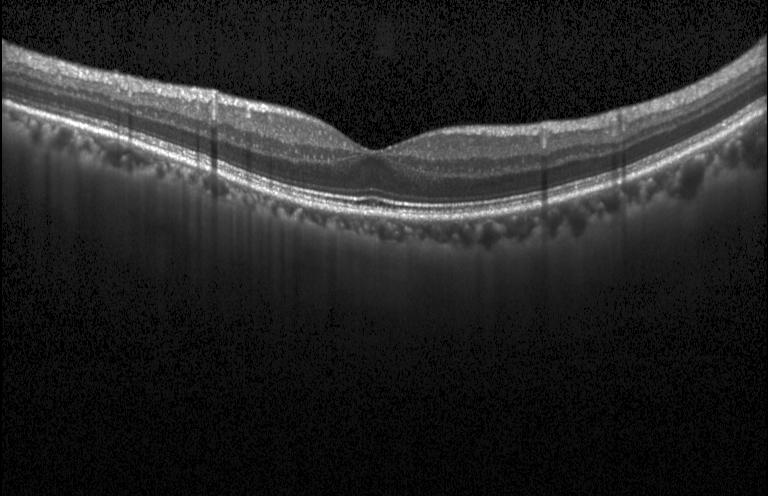 Macular OCT: no CNV, no DME, and no drusen.